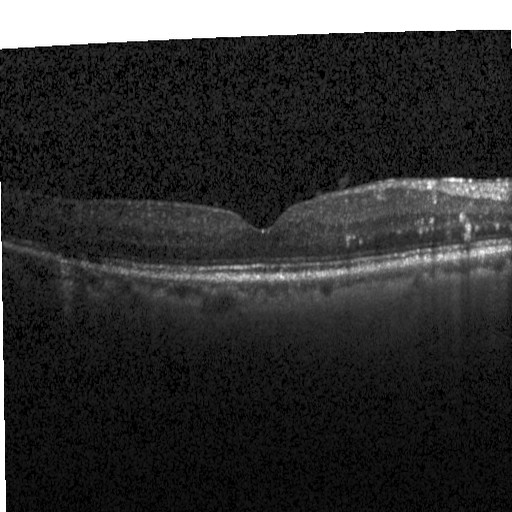
Through the macula; retinal OCT B-scan — Diagnosis: diabetic macular edema.